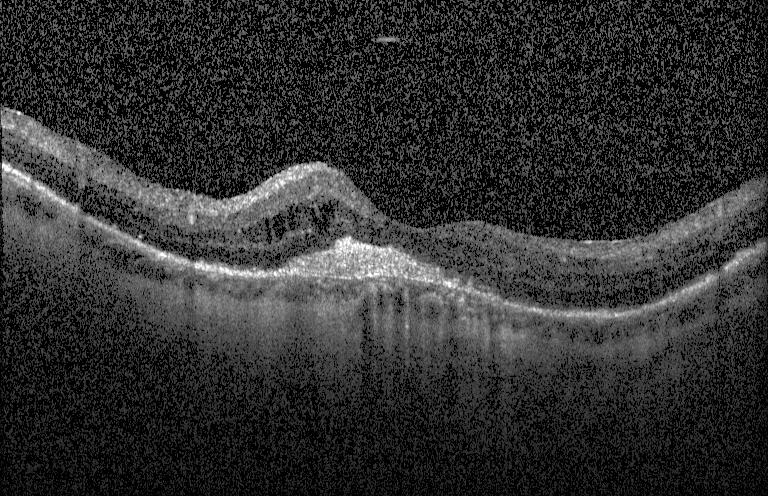

Impression: CNV.